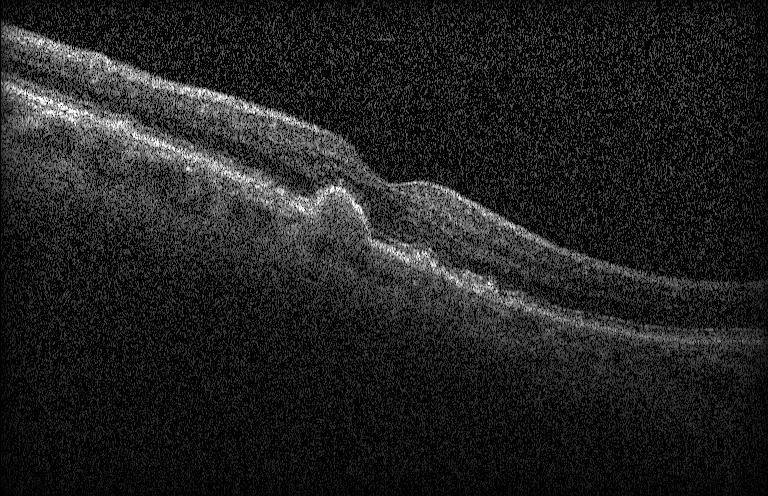

Dx: drusen.